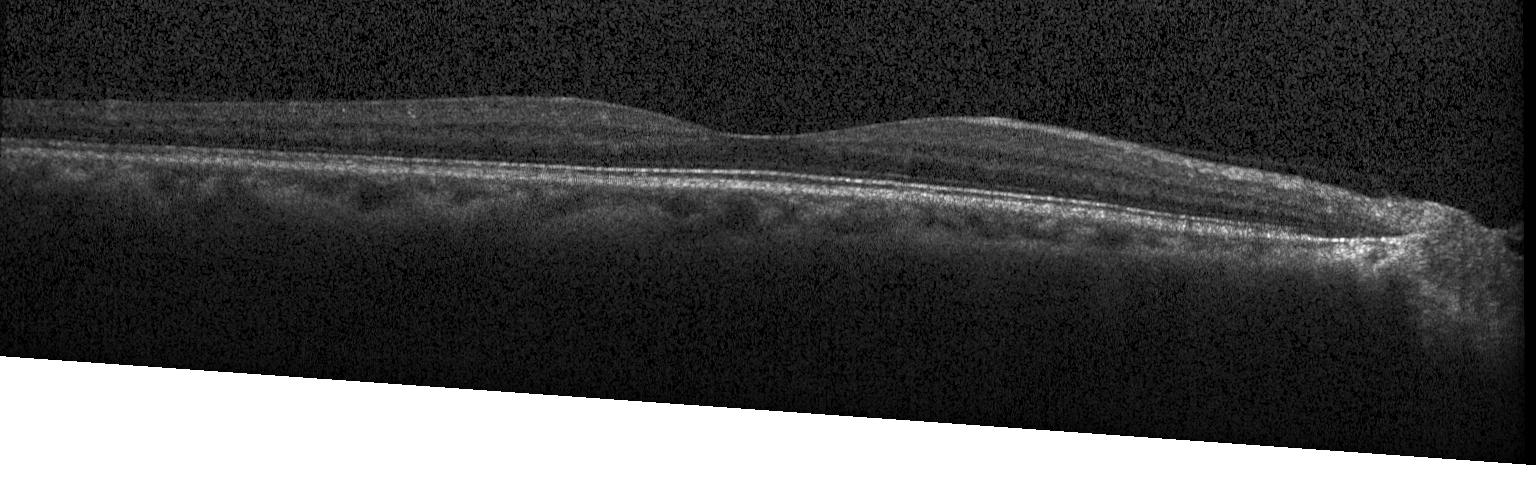 Dx: no choroidal neovascularization, no diabetic macular edema, and no drusen.